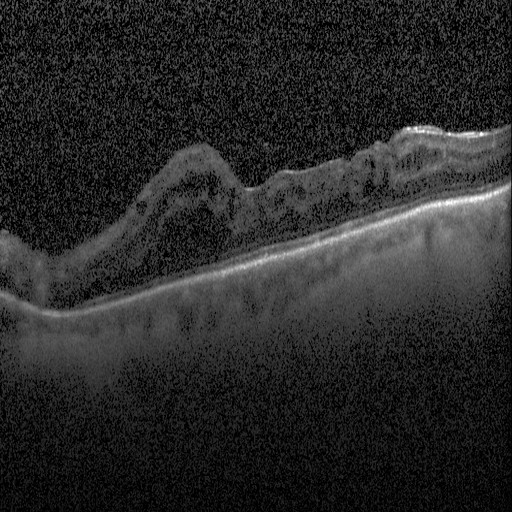

Instrument: Heidelberg Spectralis · retinal OCT cross-section.
Dx: DME.